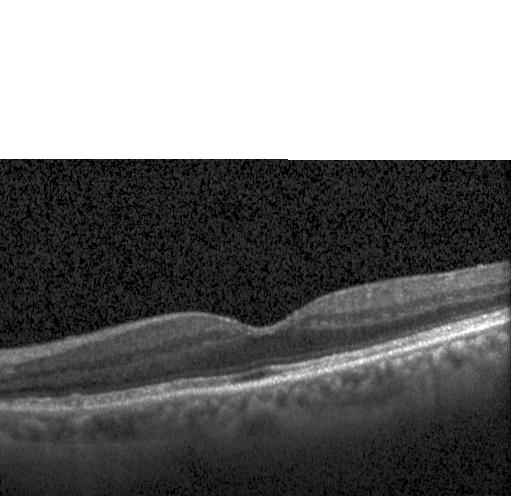
Finding: no evidence of choroidal neovascularization, diabetic macular edema, or drusen.